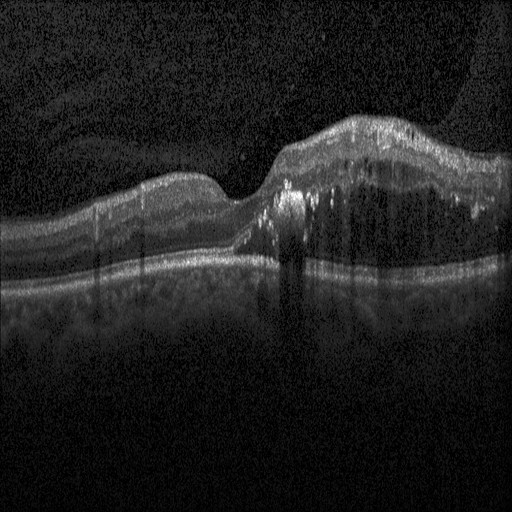

Impression: diabetic macular edema (DME).